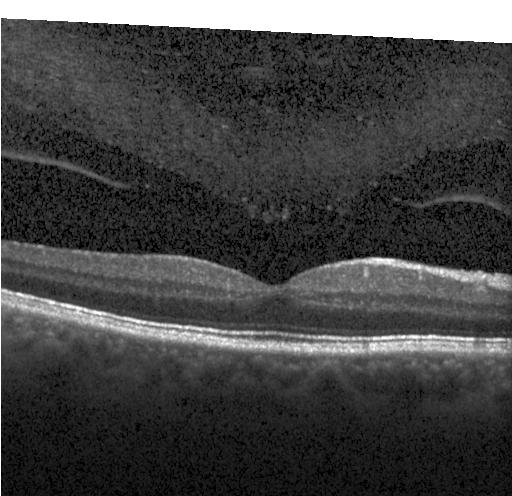

Optical coherence tomography B-scan · spectral-domain optical coherence tomography · macular scan · instrument: Heidelberg Spectralis
OCT finding: no evidence of CNV, DME, or drusen.